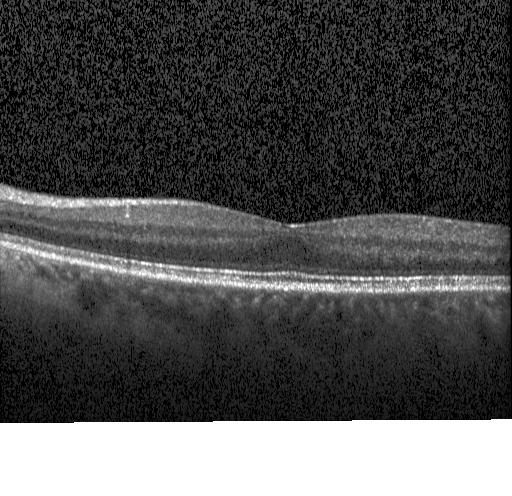
Assessment: no evidence of choroidal neovascularization, diabetic macular edema, or drusen.